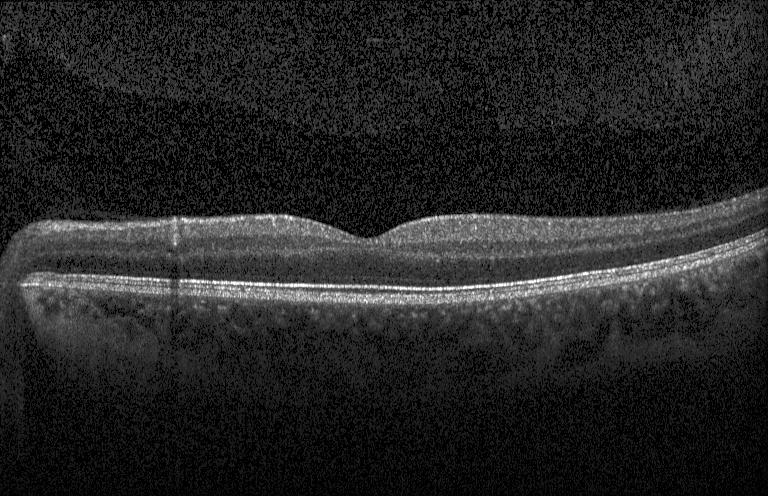

Optical coherence tomography B-scan — Dx: neither choroidal neovascularization, diabetic macular edema, nor drusen.